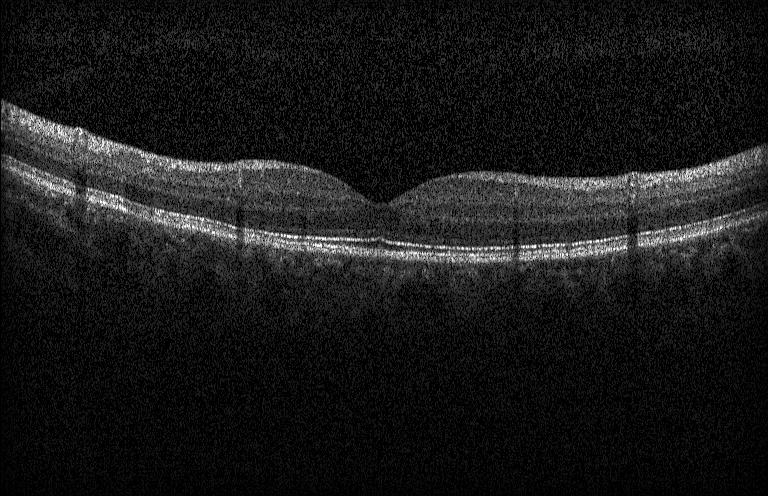
Instrument: Heidelberg Spectralis · retinal OCT B-scan · spectral-domain OCT · through the macula
Macular OCT: no CNV, no DME, and no drusen.